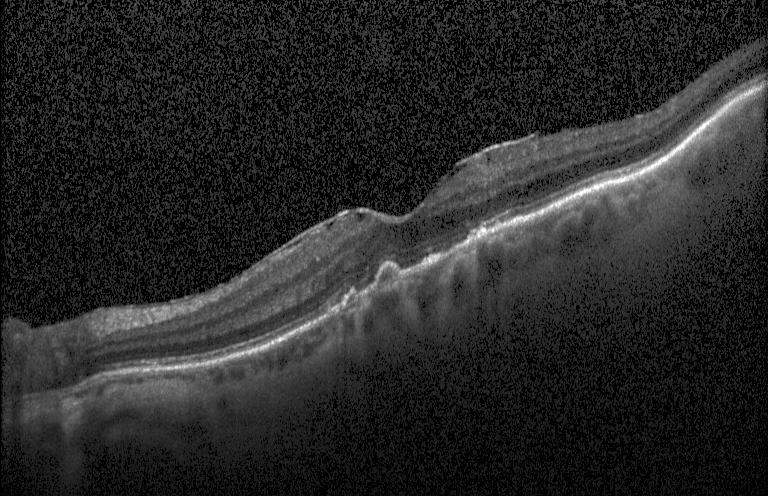

Diagnosis: multiple drusen.